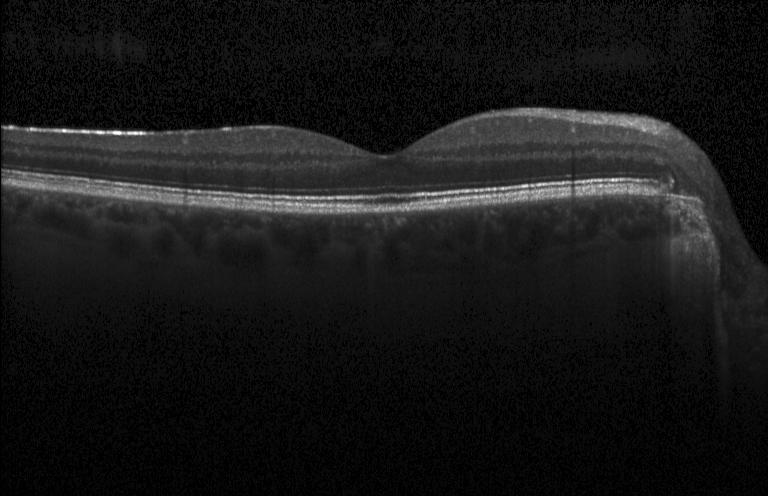
Retinal OCT cross-section, spectral-domain OCT, through the macula
No CNV, no DME, and no drusen.